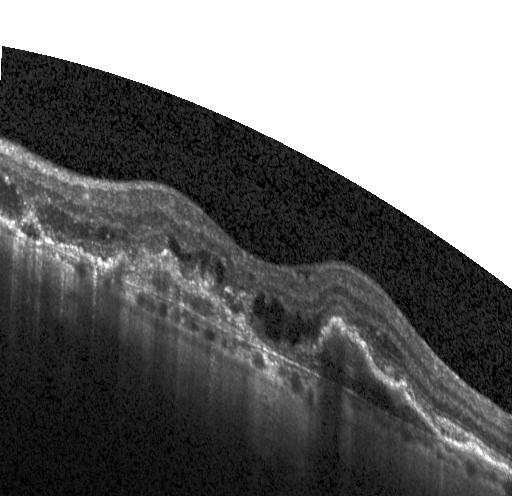

Spectral-domain OCT · optical coherence tomography B-scan · horizontal scan through the fovea · Heidelberg Spectralis — Finding: a choroidal neovascular membrane.